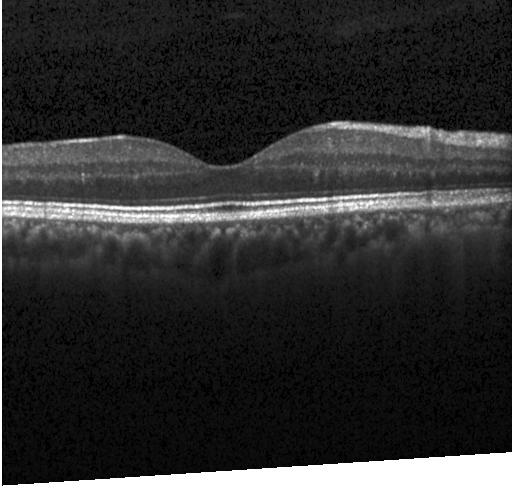

OCT B-scan showing no evidence of choroidal neovascularization, diabetic macular edema, or drusen.